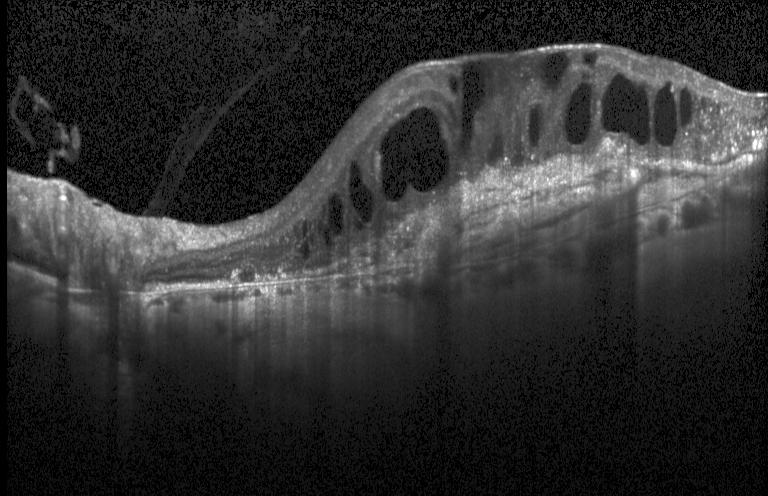 Spectral-domain OCT; retinal OCT B-scan; fovea-centered. OCT finding: a choroidal neovascular membrane.